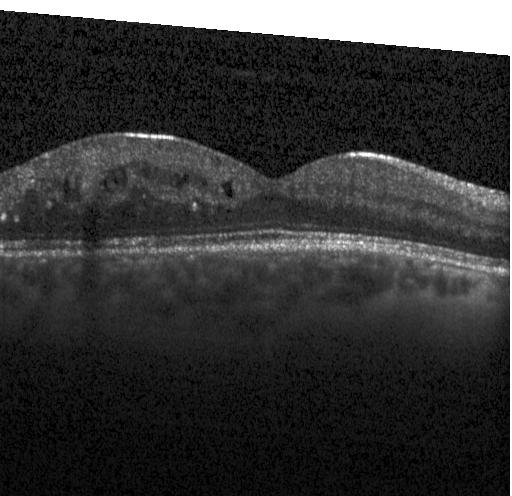
Heidelberg Spectralis OCT system, fovea-centered, optical coherence tomography B-scan, spectral-domain OCT.
Diagnosis: diabetic macular edema (DME).